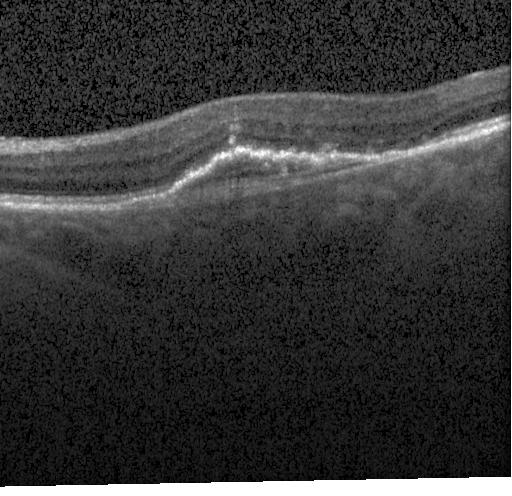 Dx: a choroidal neovascular membrane.